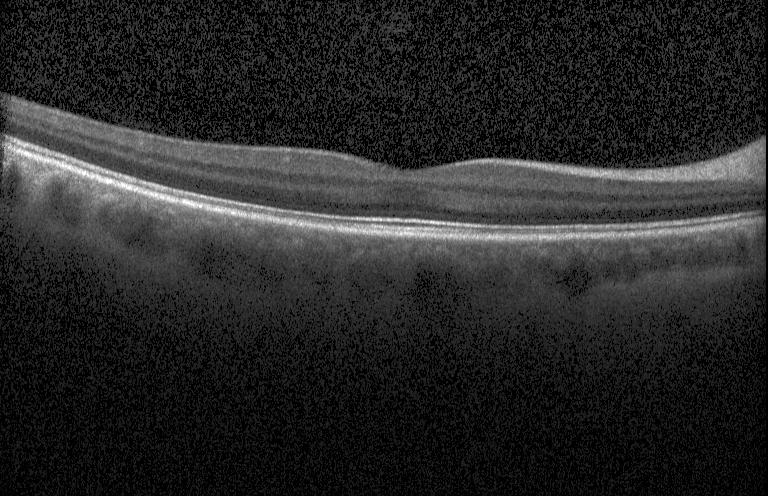 Optical coherence tomography B-scan
No CNV, DME, or drusen.